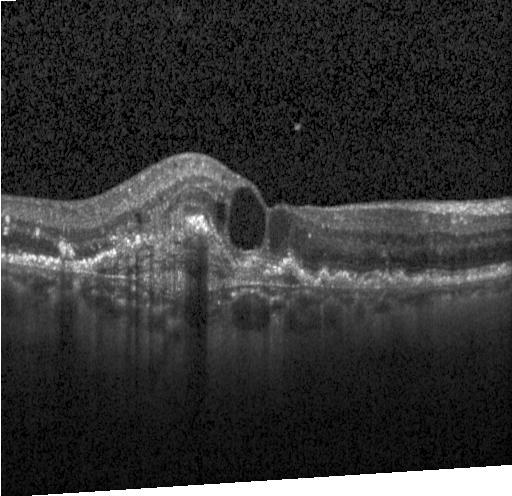
Heidelberg Spectralis, spectral-domain OCT, optical coherence tomography scan.
Dx: a choroidal neovascular membrane.